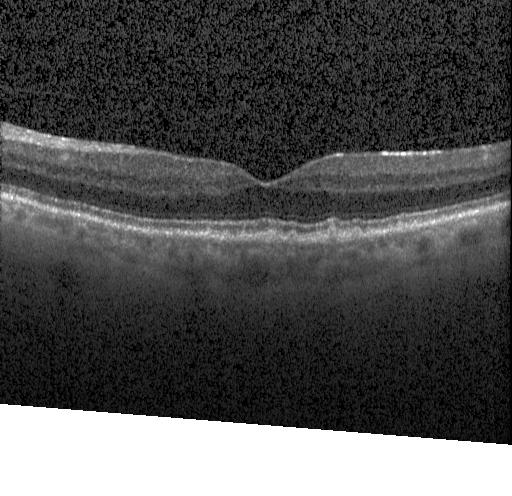
Spectral-domain OCT B-scan: drusen.